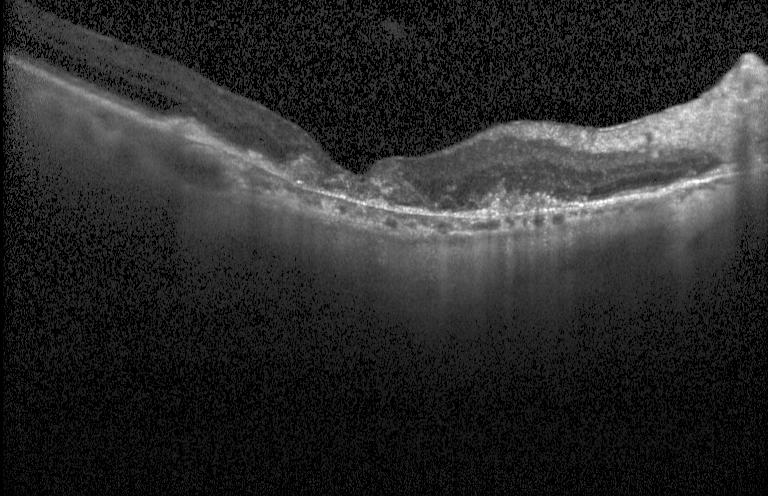
Retinal OCT cross-section showing CNV.